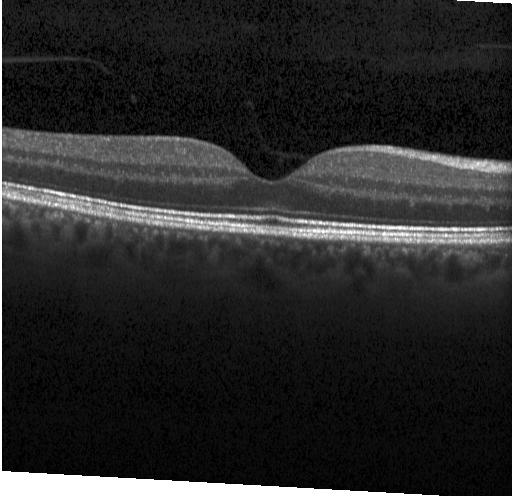 This B-scan demonstrates no choroidal neovascularization, diabetic macular edema, or drusen.